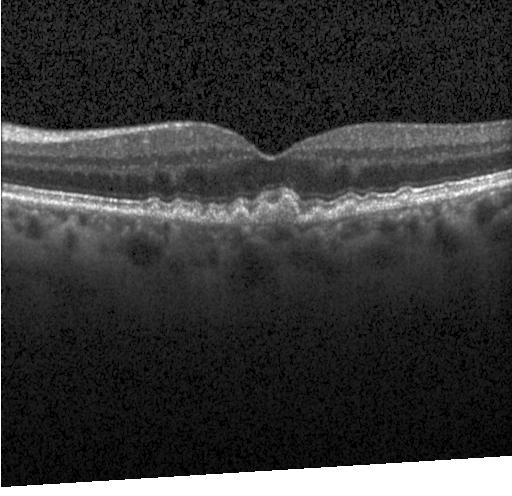
Through the macula; optical coherence tomography scan; spectral-domain optical coherence tomography. Diagnosis: sub-RPE drusenoid deposits.